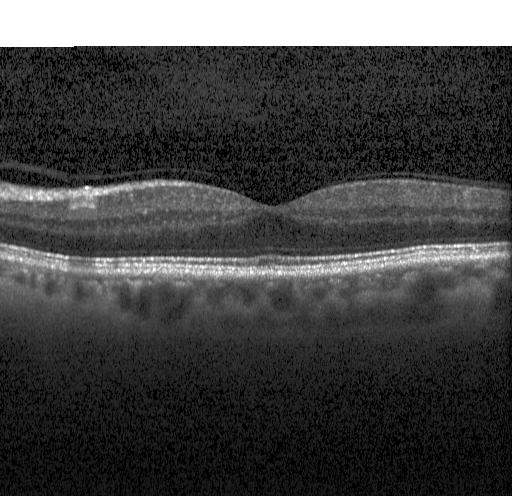
Centered on the fovea, SD-OCT, OCT B-scan.
The scan shows no choroidal neovascularization, no diabetic macular edema, and no drusen.